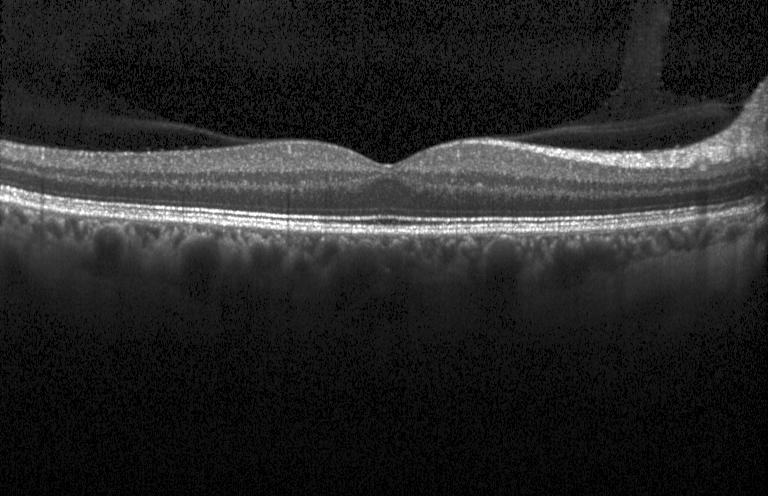 No CNV, DME, or drusen.